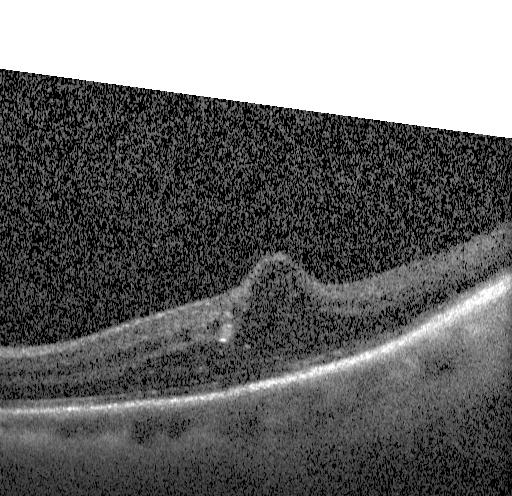
Optical coherence tomography B-scan. Spectral-domain OCT.
Impression: diabetic macular edema (DME).